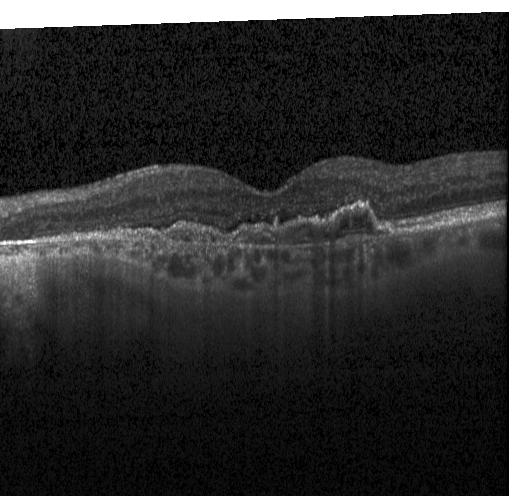 OCT line scan · SD-OCT. Dx: a choroidal neovascular membrane.